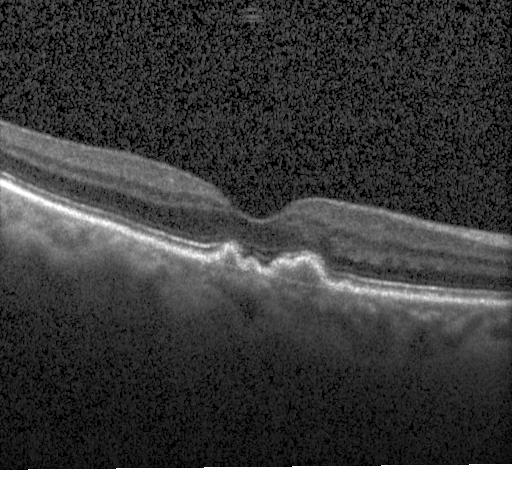
Retinal OCT B-scan. This B-scan demonstrates drusen.